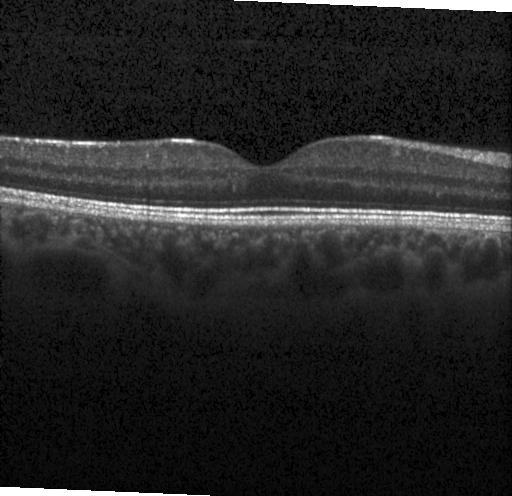
Retinal OCT cross-section showing no evidence of CNV, DME, or drusen.